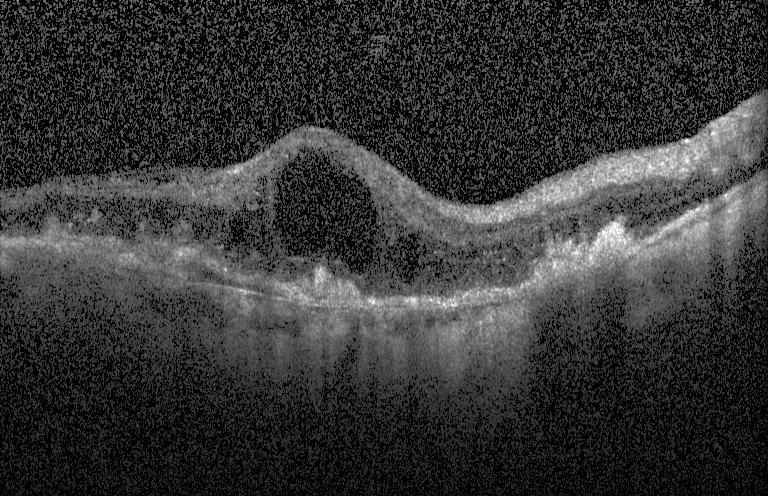

Macular scan · Heidelberg Spectralis · retinal OCT B-scan.
Impression: CNV.